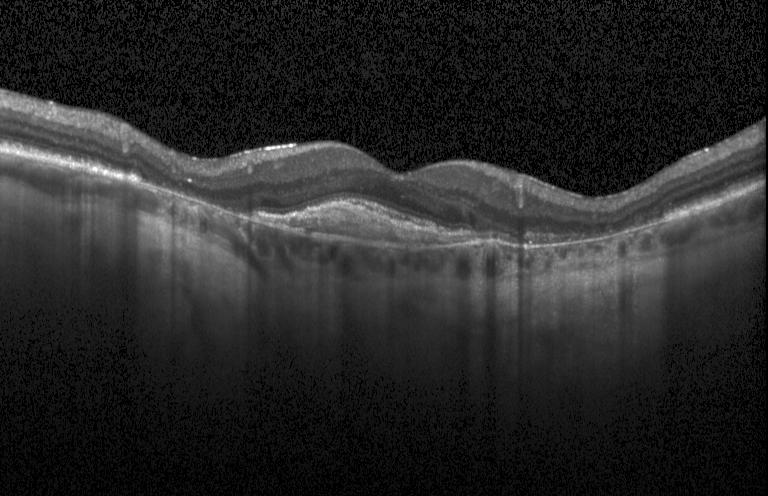 Retinal OCT cross-section.
Finding: a choroidal neovascular membrane.